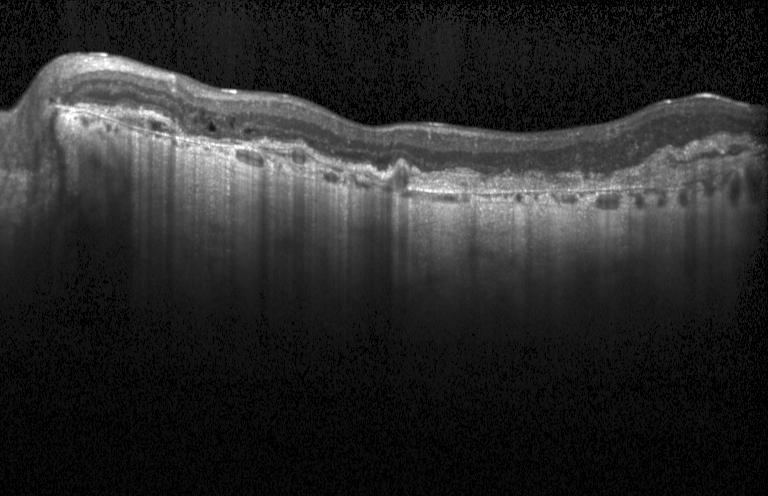

Macular scan. Spectral-domain optical coherence tomography. OCT B-scan. Instrument: Heidelberg Spectralis
Finding: choroidal neovascularization.